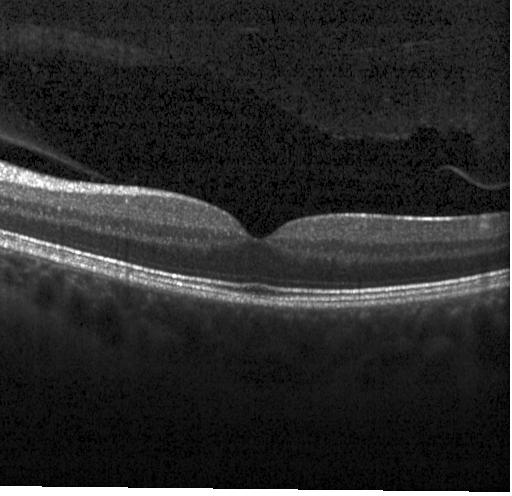

Spectral-domain OCT B-scan: no evidence of choroidal neovascularization, diabetic macular edema, or drusen.